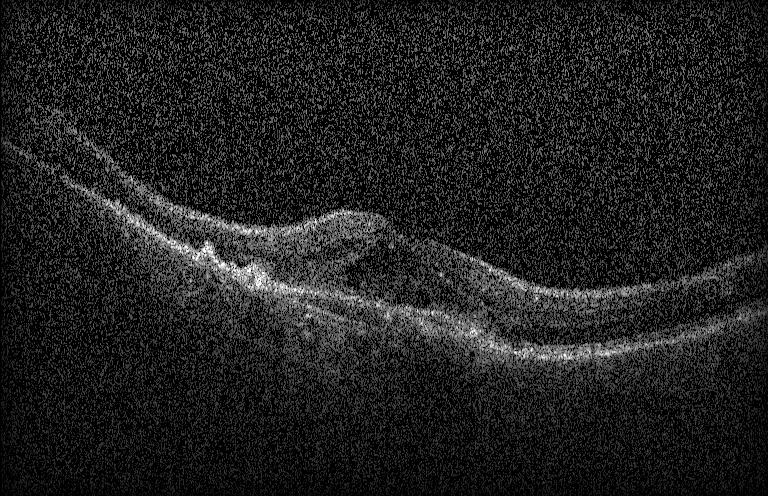 Acquired on a Heidelberg Spectralis, through the macula, retinal OCT B-scan. CNV.